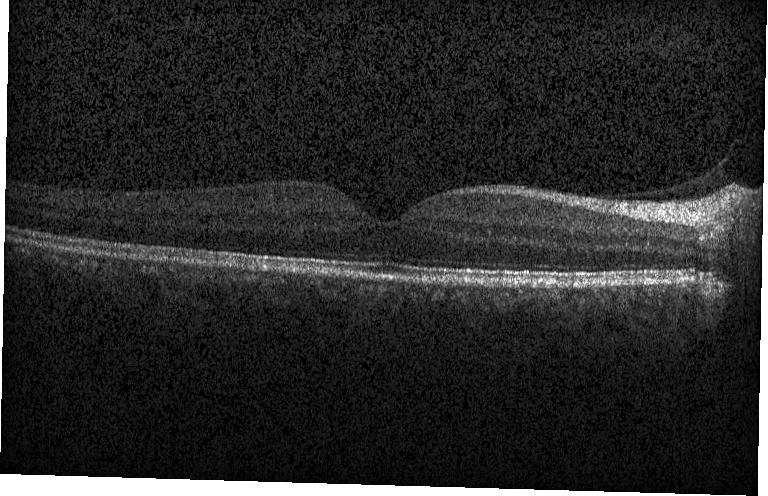

Horizontal scan through the fovea. Retinal OCT cross-section. Instrument: Heidelberg Spectralis. SD-OCT — Finding: neither choroidal neovascularization, diabetic macular edema, nor drusen.